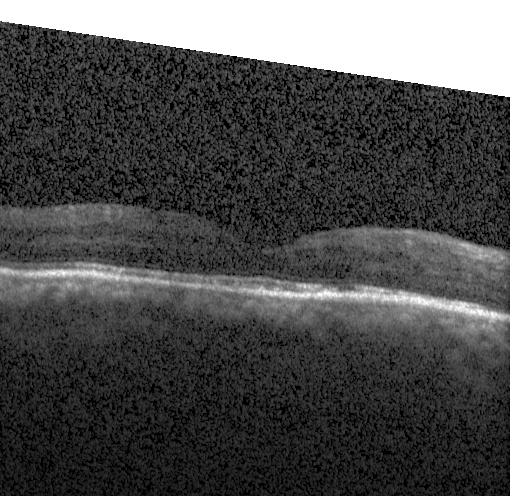

Retinal OCT cross-section.
Dx: neither choroidal neovascularization, diabetic macular edema, nor drusen.